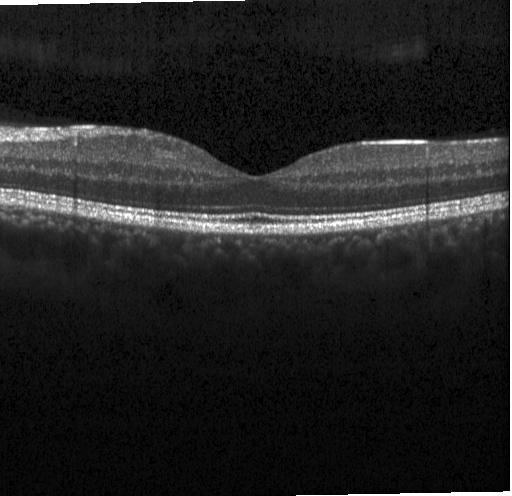 Heidelberg Spectralis, retinal OCT B-scan. Assessment: no CNV, no DME, and no drusen.